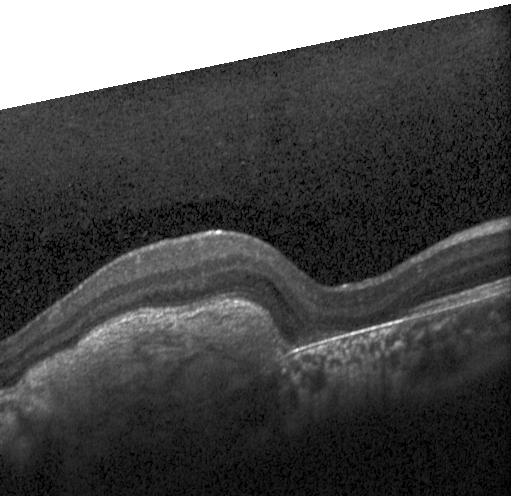

OCT line scan, SD-OCT, Heidelberg Spectralis — Finding: choroidal neovascularization (CNV).